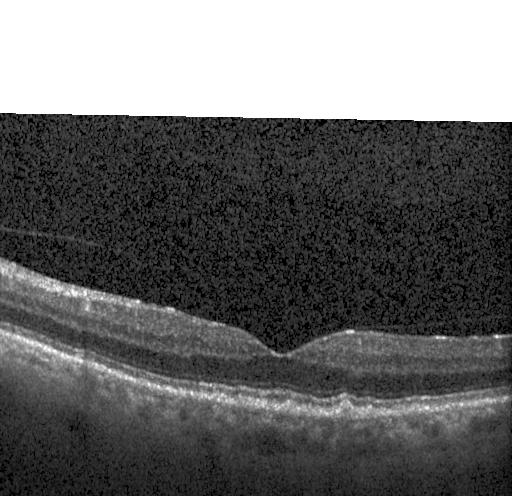 Finding: drusen.